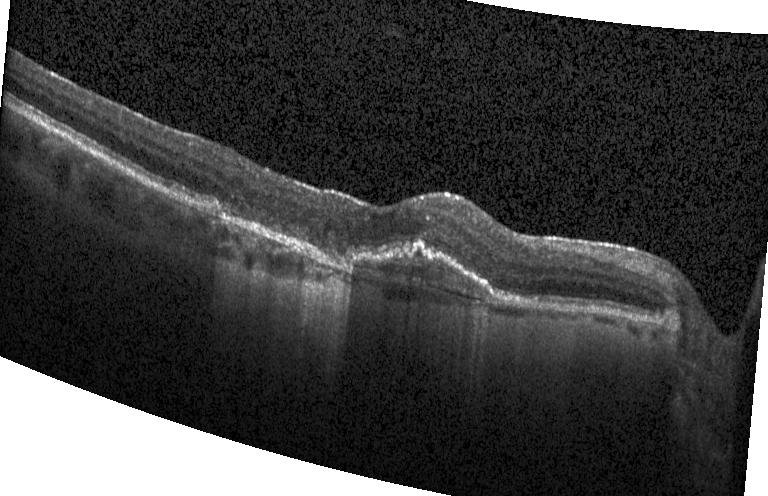

Acquired on a Heidelberg Spectralis; retinal OCT cross-section; spectral-domain OCT.
OCT finding: a choroidal neovascular membrane.